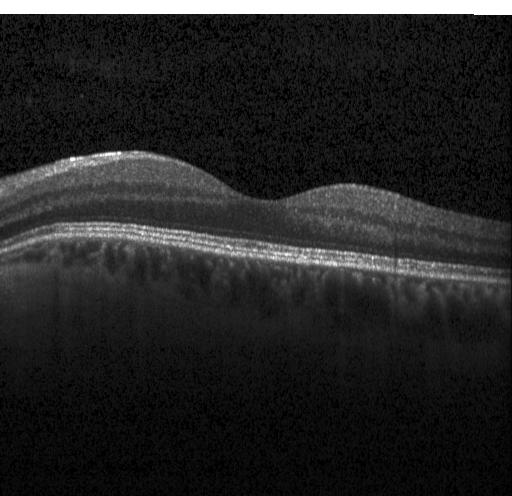
Optical coherence tomography B-scan · spectral-domain OCT — OCT finding: no CNV, DME, or drusen.